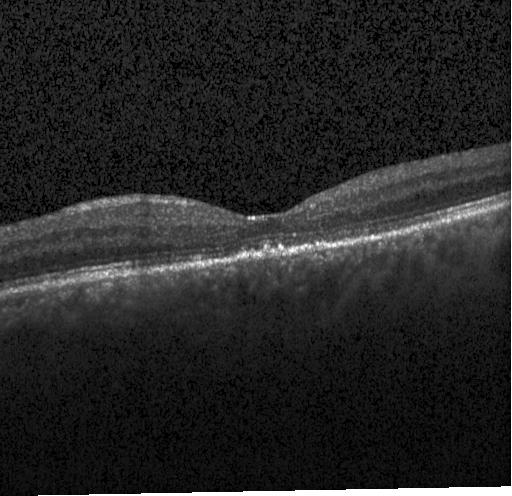

OCT finding: sub-RPE drusenoid deposits.